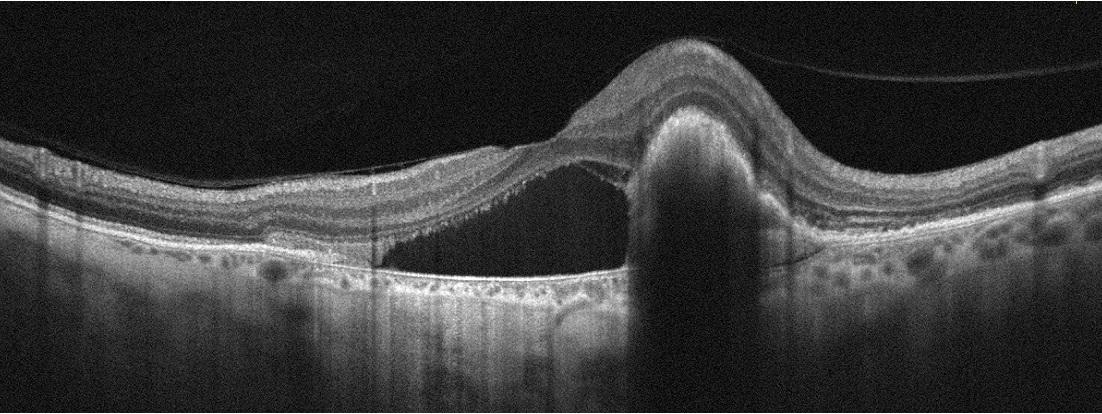
Optovue Avanti RTVue XR · retinal OCT B-scan — OCT finding: AMD.